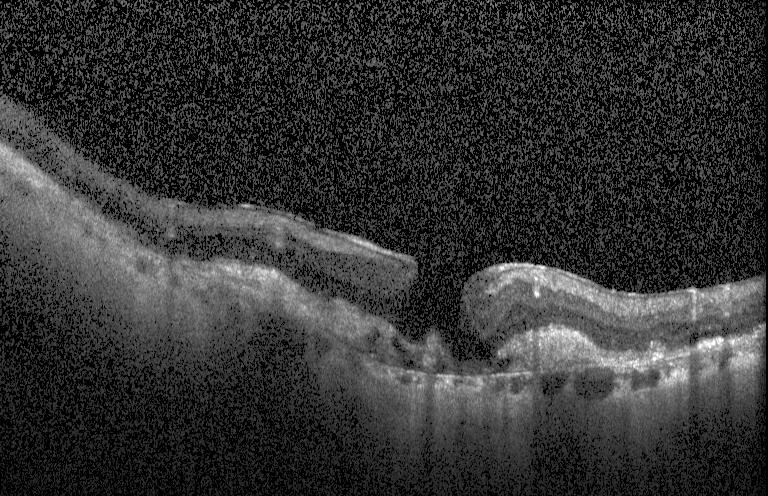

Impression: choroidal neovascularization.